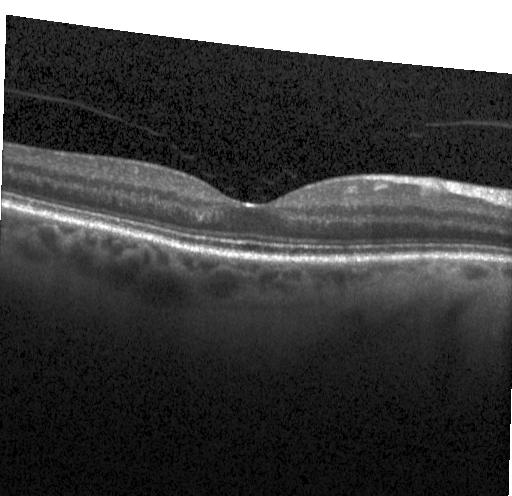
Spectral-domain OCT B-scan: neither choroidal neovascularization, diabetic macular edema, nor drusen.